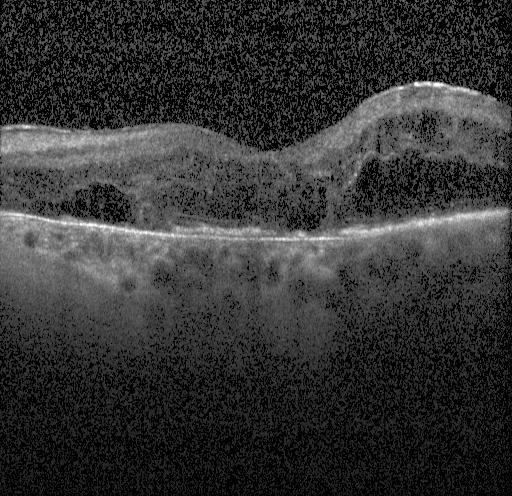
This B-scan demonstrates choroidal neovascularization.